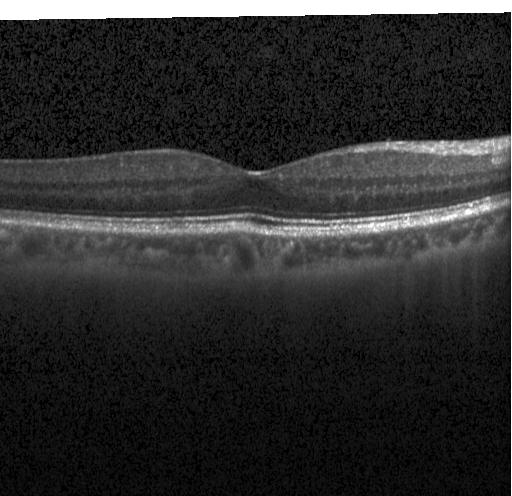
Fovea-centered. Optical coherence tomography B-scan. Heidelberg Spectralis OCT system
Diagnosis: no CNV, no DME, and no drusen.